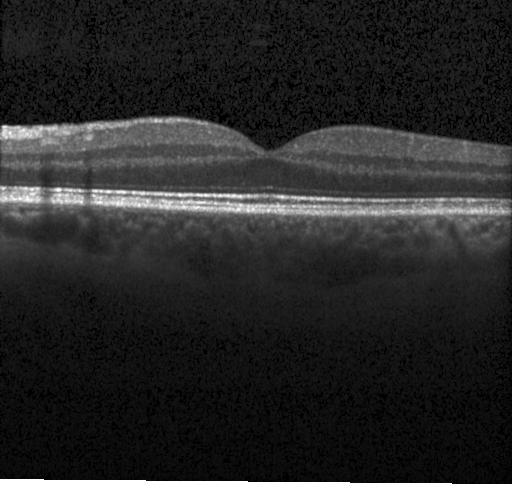

Neither choroidal neovascularization, diabetic macular edema, nor drusen.